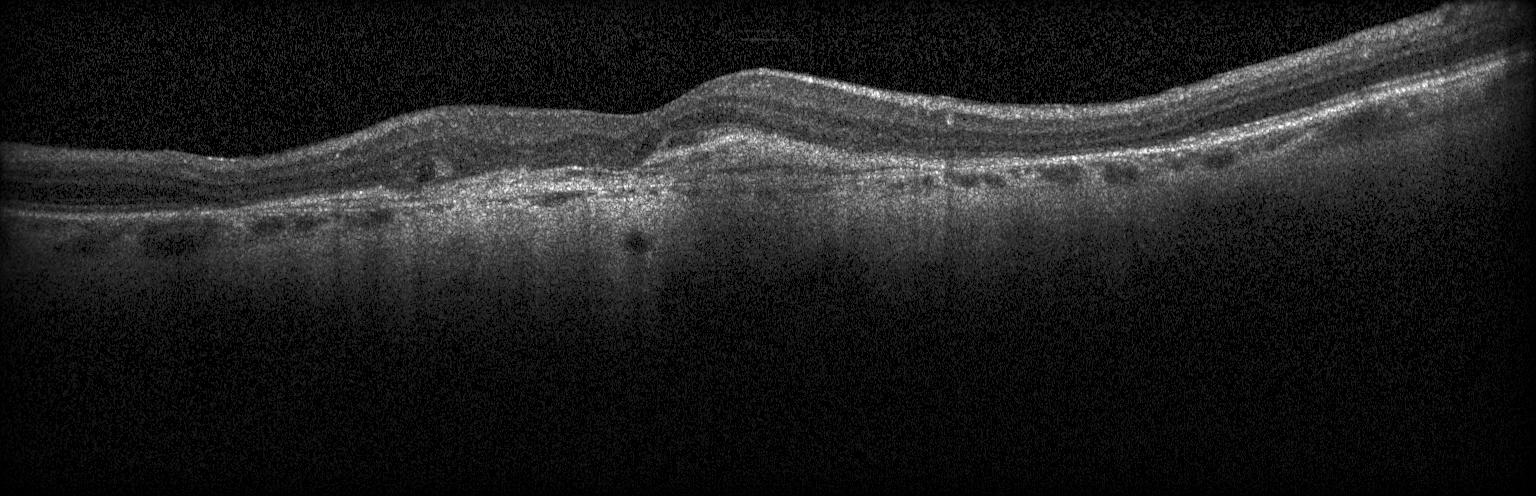
The scan shows choroidal neovascularization.